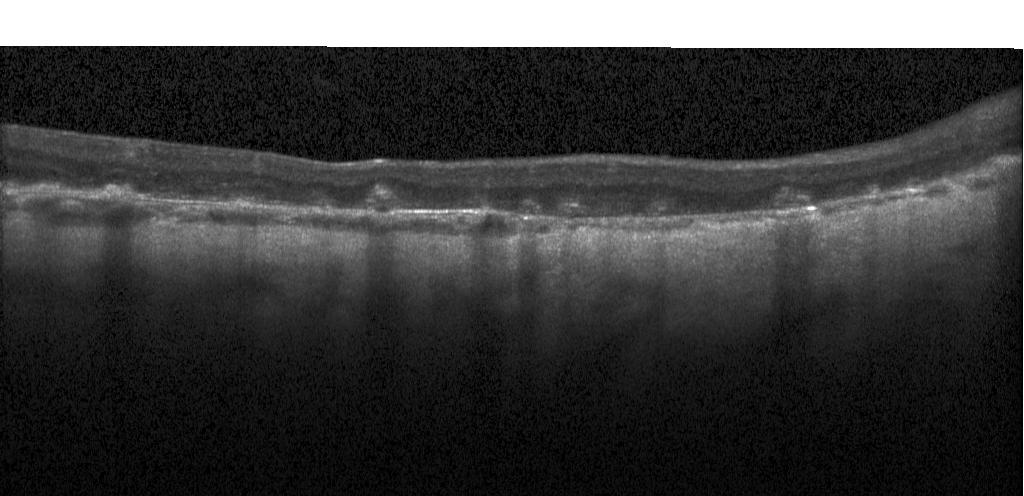

Macular OCT: neither choroidal neovascularization, diabetic macular edema, nor drusen.